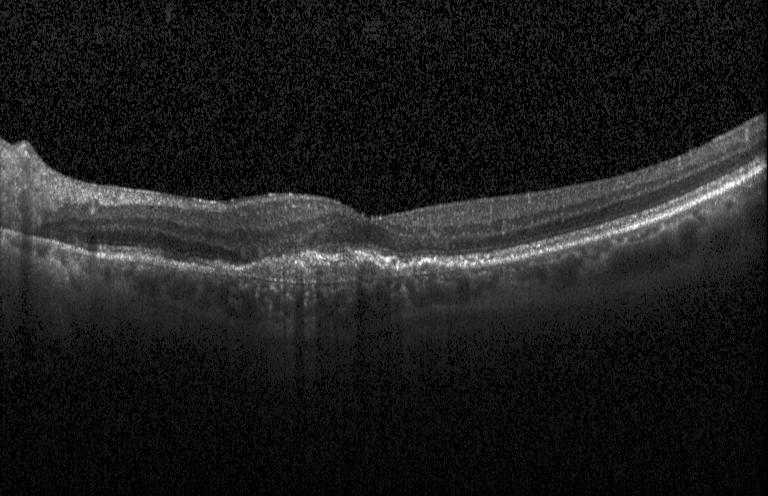

Spectral-domain OCT · Heidelberg Spectralis · optical coherence tomography B-scan.
Impression: choroidal neovascularization.